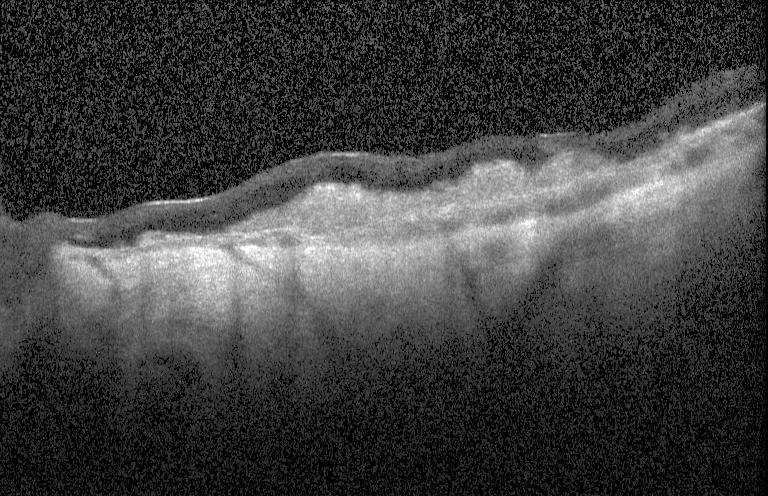 Acquired on a Heidelberg Spectralis, through the macula, OCT line scan. This B-scan demonstrates choroidal neovascularization.